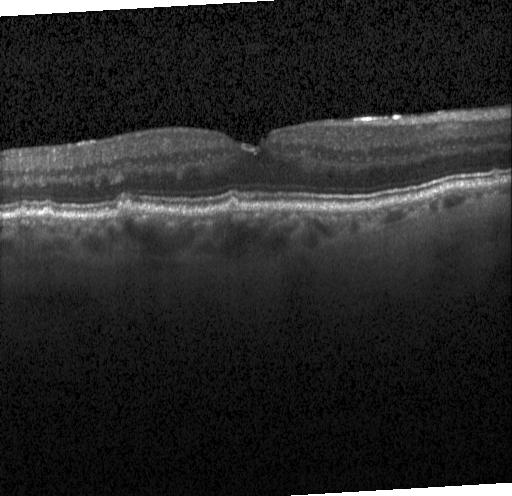
OCT scan showing drusen.